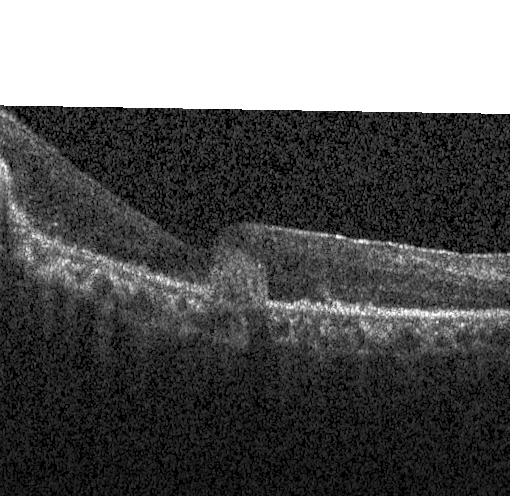

Finding: a choroidal neovascular membrane.